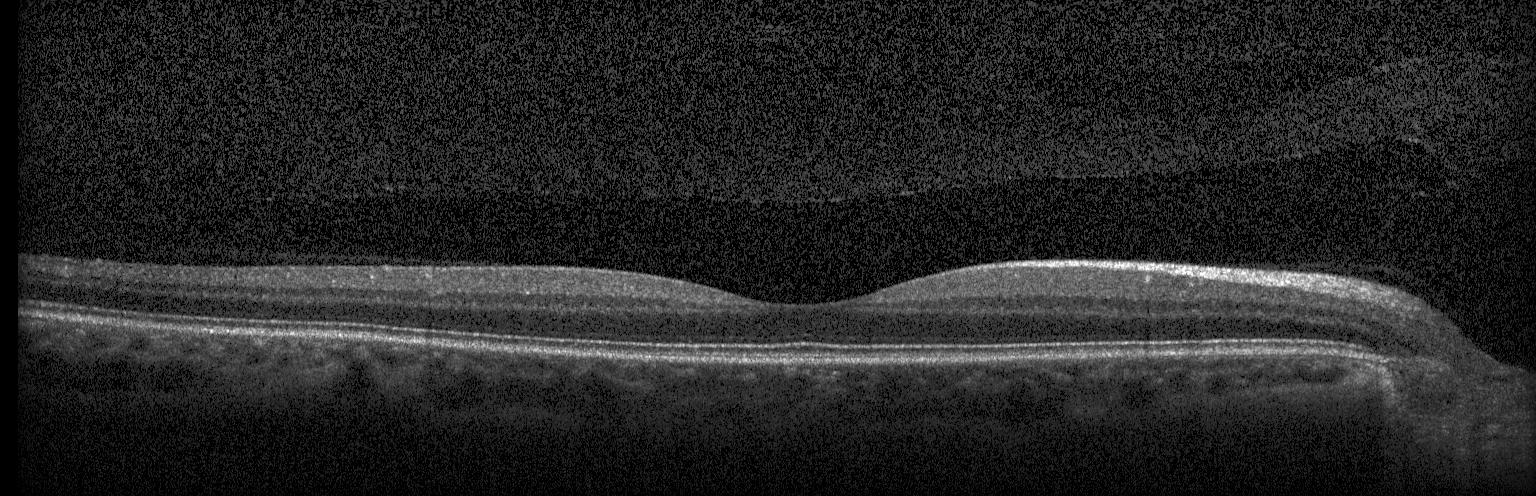
Acquired on a Heidelberg Spectralis, OCT line scan, through the macula. OCT finding: no evidence of CNV, DME, or drusen.